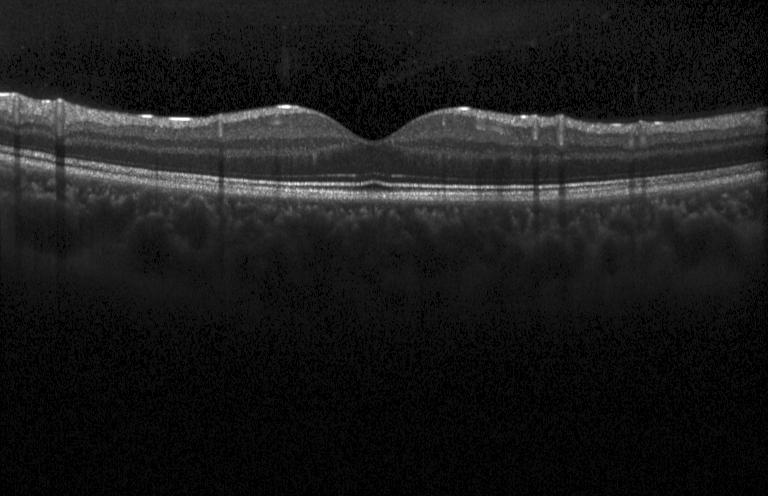

Instrument: Heidelberg Spectralis; horizontal scan through the fovea; spectral-domain optical coherence tomography; OCT line scan.
Finding: no evidence of choroidal neovascularization, diabetic macular edema, or drusen.